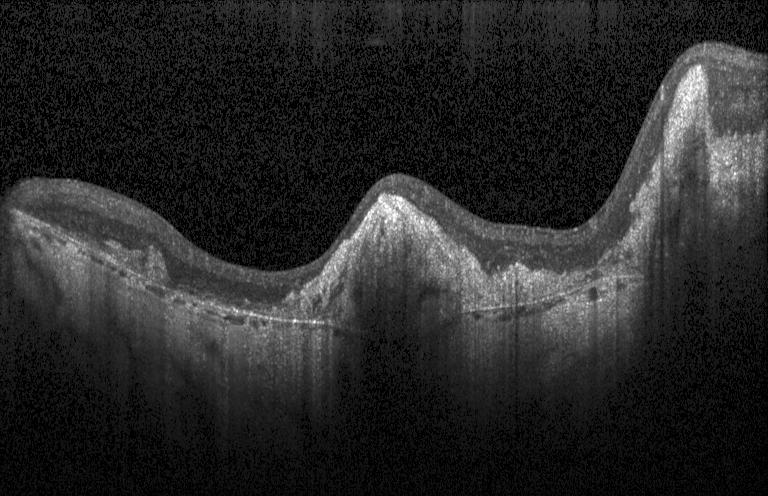

Acquired on a Heidelberg Spectralis; spectral-domain OCT; optical coherence tomography scan.
Macular OCT: a choroidal neovascular membrane.